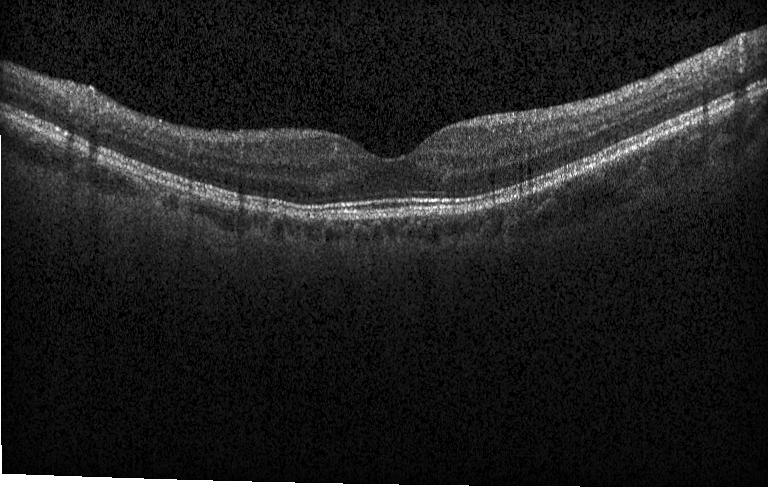
OCT B-scan showing no evidence of CNV, DME, or drusen.